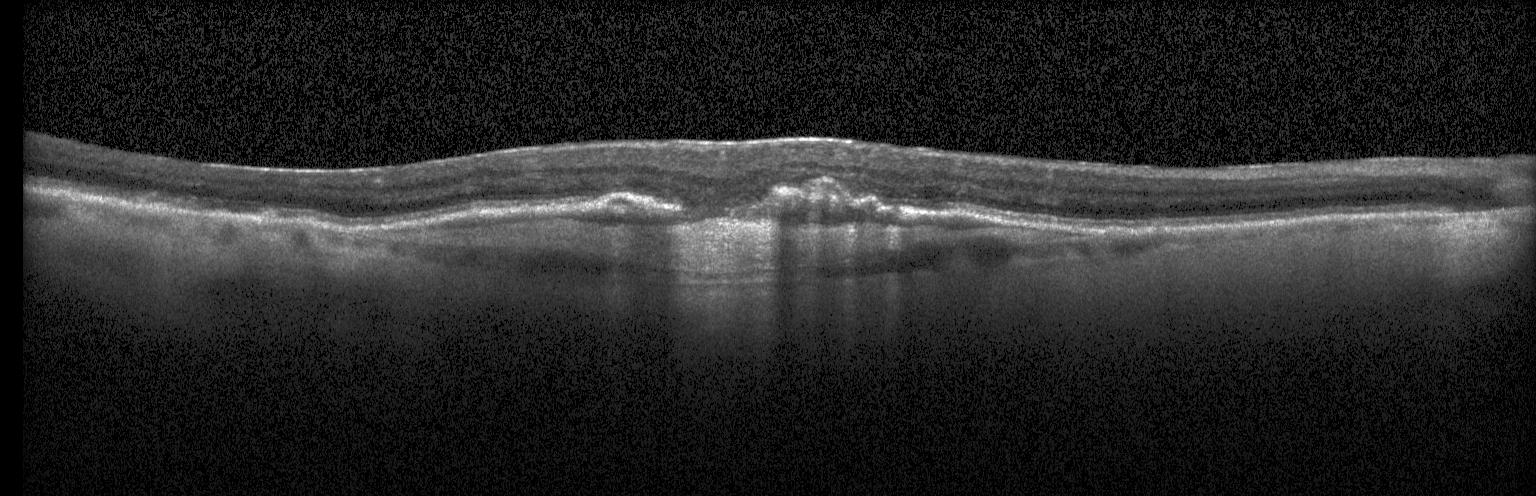 Retinal OCT B-scan, through the macula, Heidelberg Spectralis, spectral-domain optical coherence tomography. A choroidal neovascular membrane.